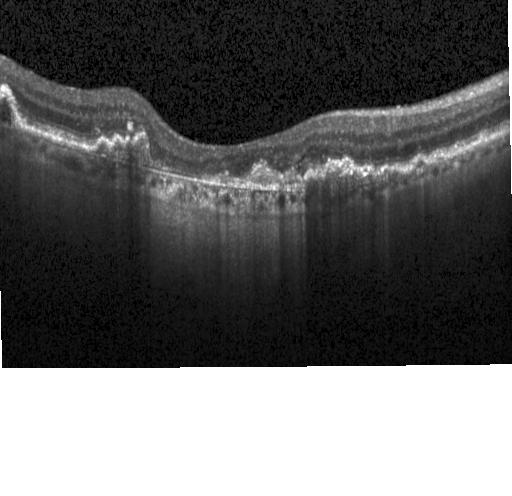

Impression: a choroidal neovascular membrane.